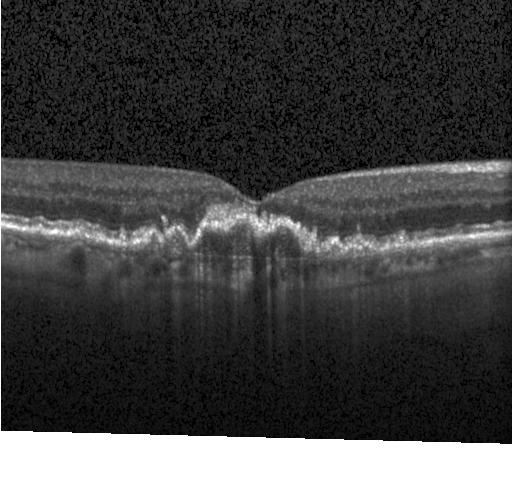

Through the macula · optical coherence tomography scan · Heidelberg Spectralis
Finding: a choroidal neovascular membrane.